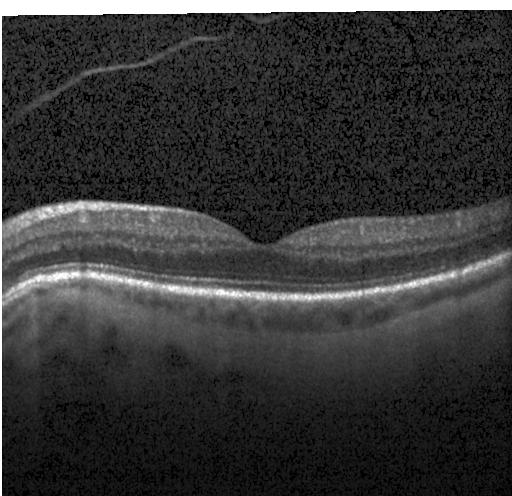
Macular OCT demonstrating no choroidal neovascularization, no diabetic macular edema, and no drusen.